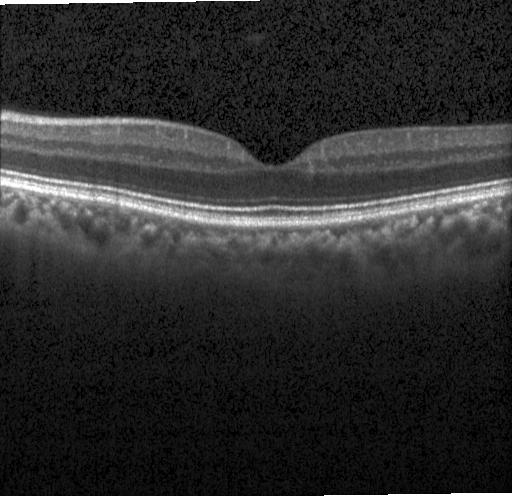
Heidelberg Spectralis · through the macula · OCT line scan — No evidence of choroidal neovascularization, diabetic macular edema, or drusen.